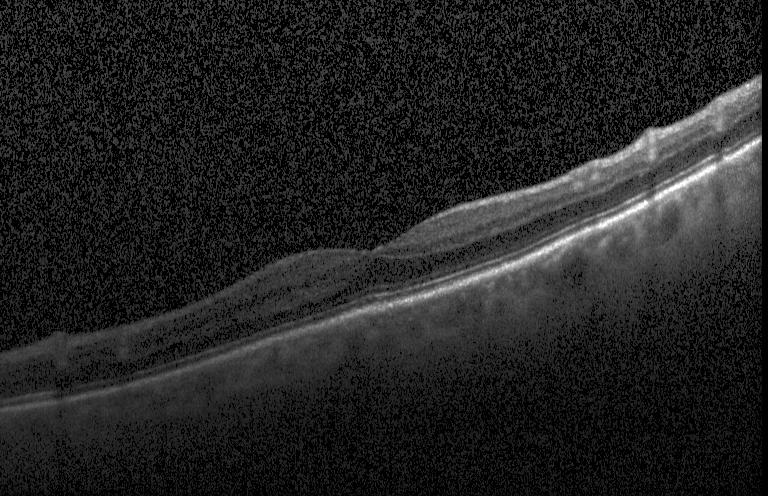

Instrument: Heidelberg Spectralis. OCT B-scan. Through the macula. The scan shows neither CNV, DME, nor drusen.